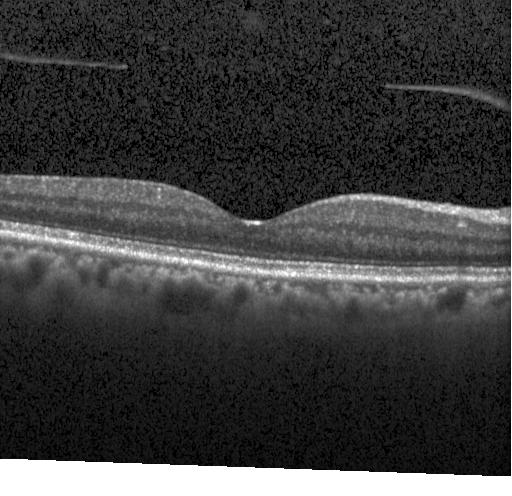
Heidelberg Spectralis OCT system; retinal OCT cross-section; horizontal scan through the fovea. The scan shows no evidence of CNV, DME, or drusen.